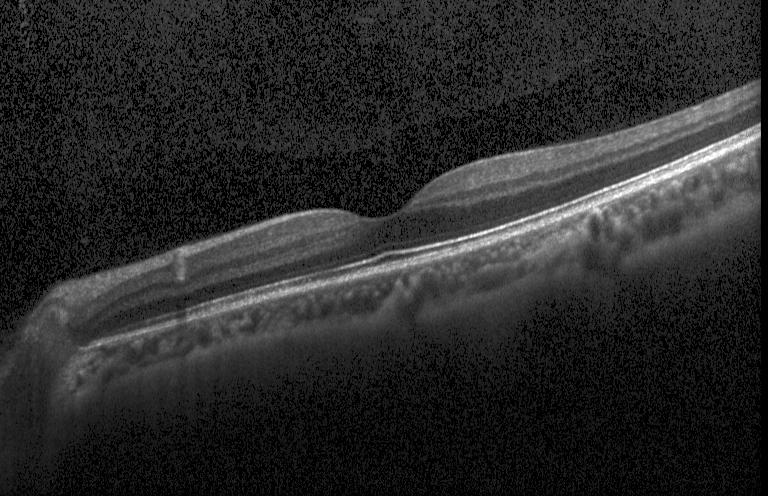

OCT line scan, acquired on a Heidelberg Spectralis — Finding: no evidence of choroidal neovascularization, diabetic macular edema, or drusen.